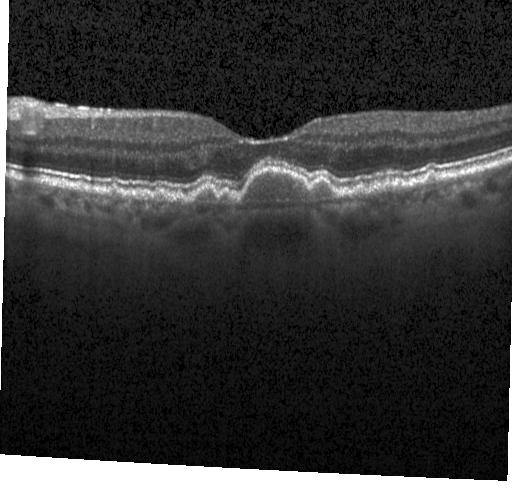 Heidelberg Spectralis OCT system. Optical coherence tomography B-scan.
This B-scan demonstrates multiple drusen.